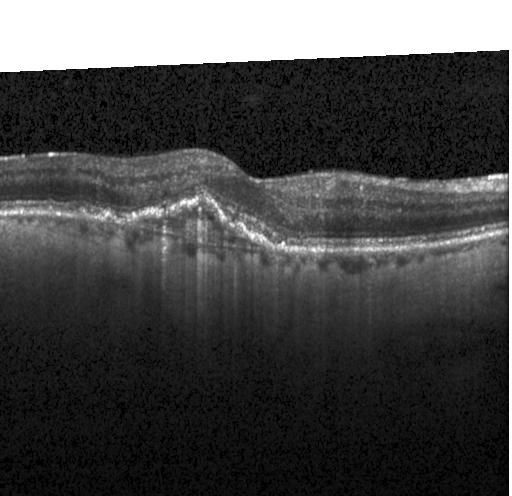
Impression: choroidal neovascularization (CNV).